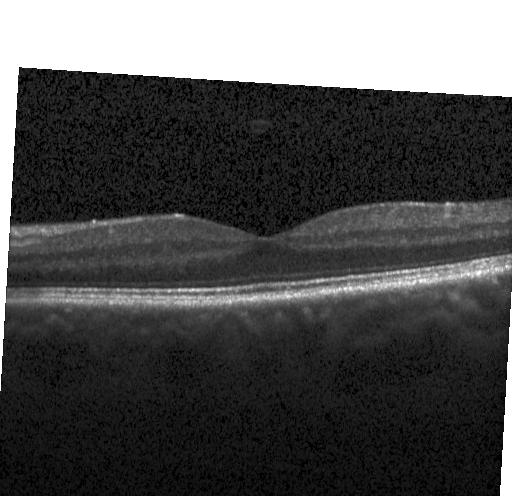

The scan shows no choroidal neovascularization, diabetic macular edema, or drusen.